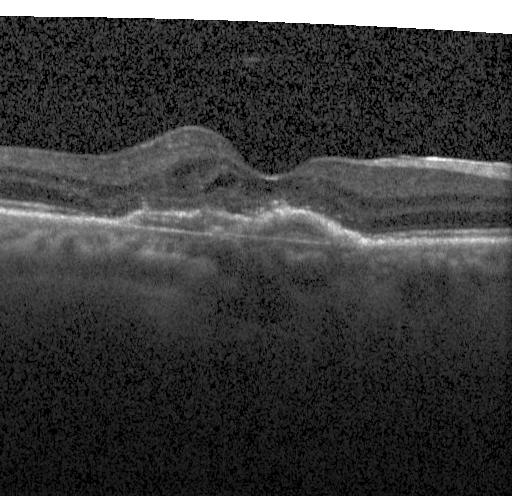

Retinal OCT B-scan · spectral-domain OCT — A choroidal neovascular membrane.